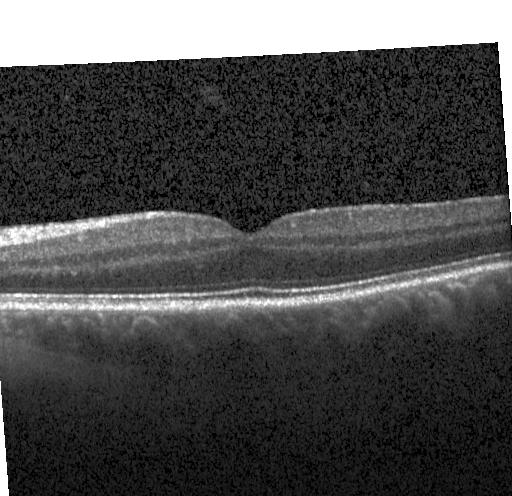 OCT line scan — Impression: no choroidal neovascularization, no diabetic macular edema, and no drusen.